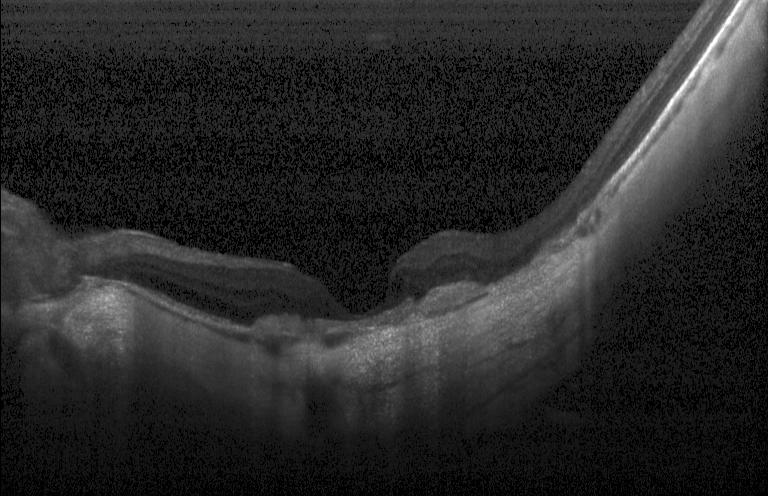
Impression: choroidal neovascularization (CNV).